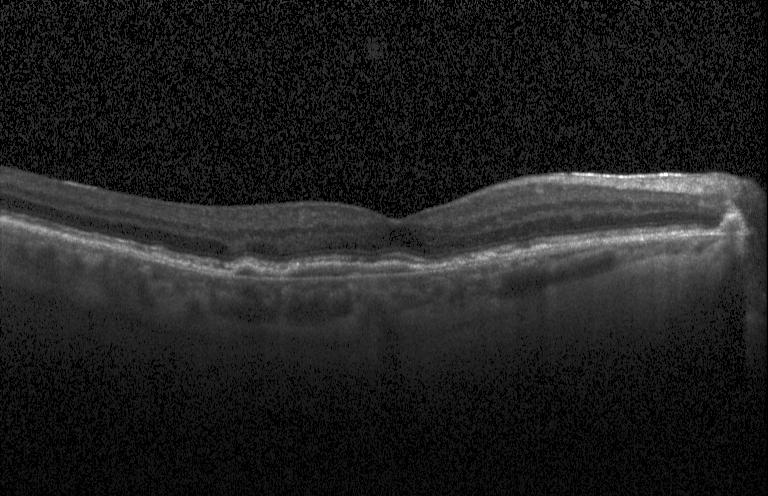

Macular scan · Heidelberg Spectralis OCT system · optical coherence tomography B-scan. Diagnosis: choroidal neovascularization.